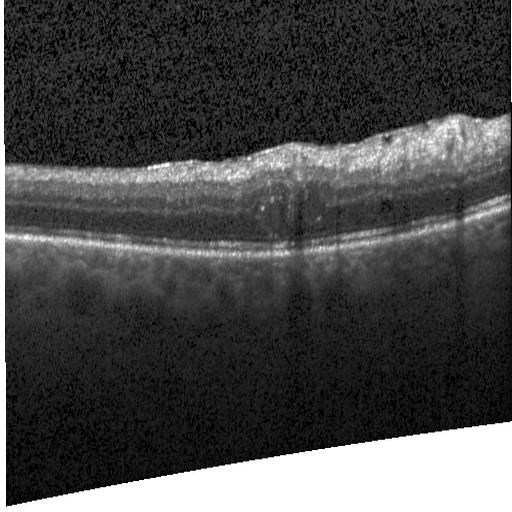 OCT B-scan · spectral-domain optical coherence tomography — Impression: diabetic macular edema (DME).